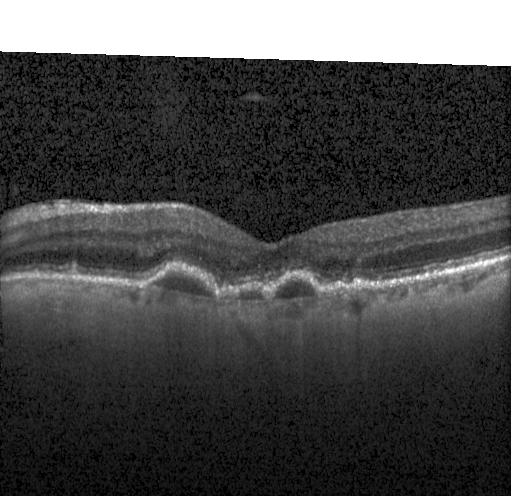

Spectral-domain OCT. Acquired on a Heidelberg Spectralis. Through the macula. Retinal OCT cross-section. The scan shows CNV.